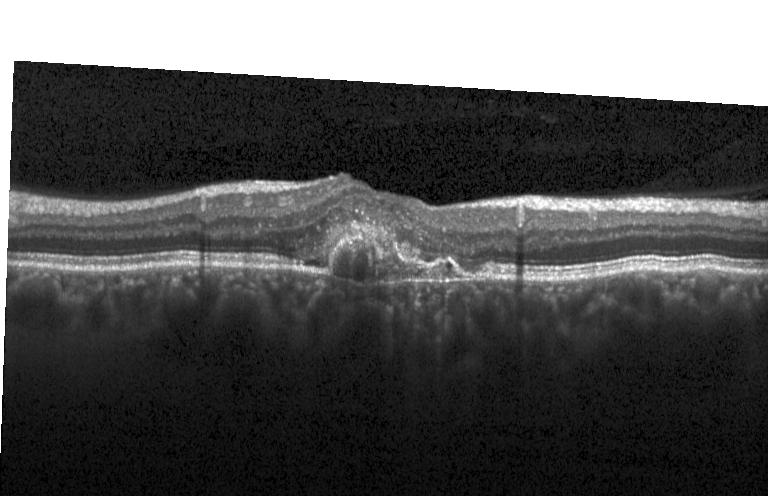
Diagnosis: choroidal neovascularization (CNV).